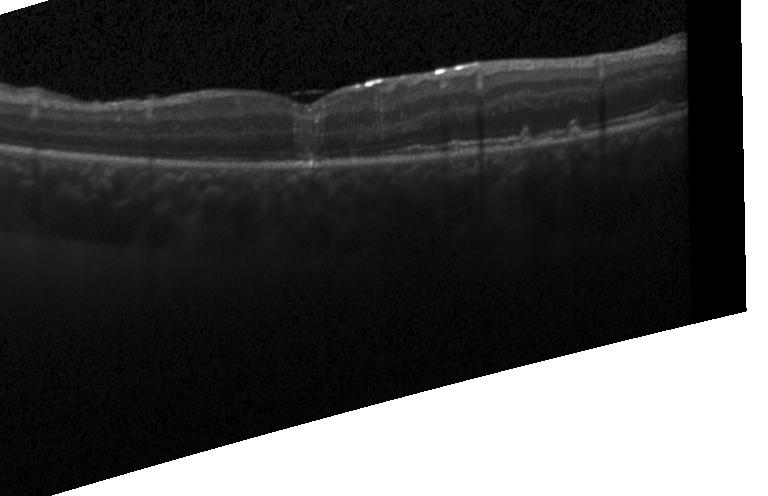 Centered on the fovea. Spectral-domain OCT. Optical coherence tomography scan
Diagnosis: multiple drusen.